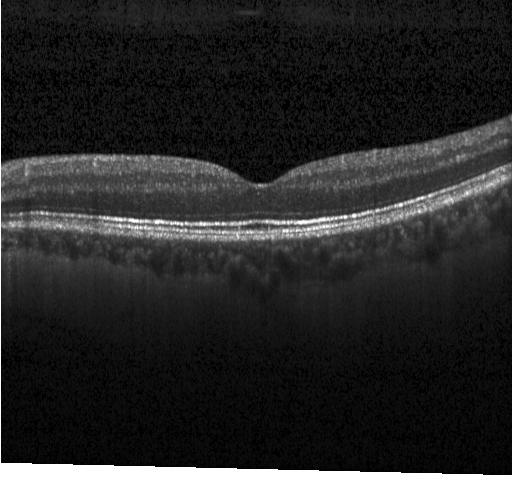

Acquired on a Heidelberg Spectralis. OCT line scan. Centered on the fovea.
Impression: neither choroidal neovascularization, diabetic macular edema, nor drusen.